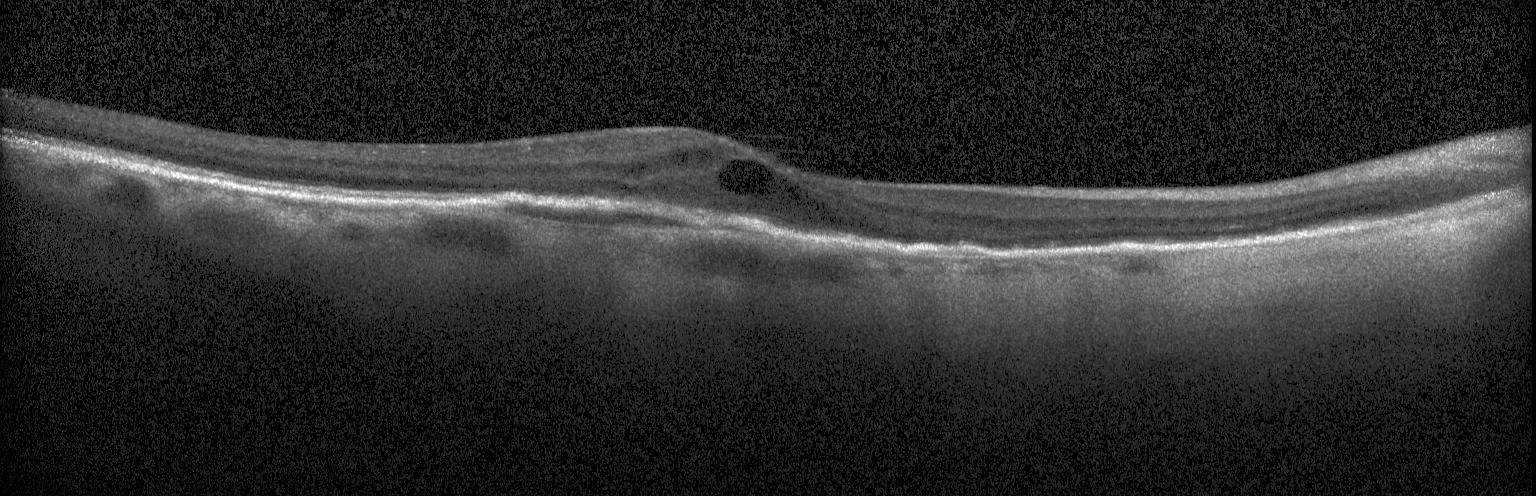

Macular OCT: choroidal neovascularization.